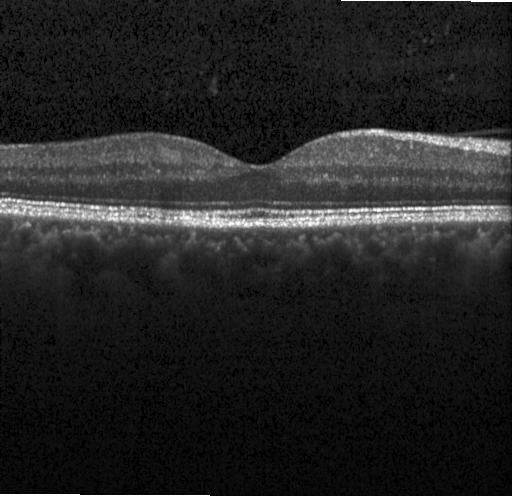
Retinal OCT cross-section. Through the macula — Diagnosis: no evidence of choroidal neovascularization, diabetic macular edema, or drusen.